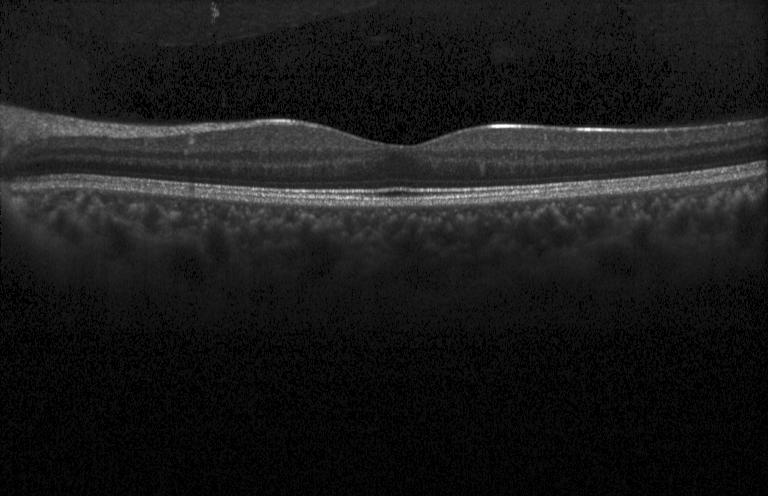 Optical coherence tomography scan · spectral-domain optical coherence tomography · acquired on a Heidelberg Spectralis · through the macula. This B-scan demonstrates no choroidal neovascularization, diabetic macular edema, or drusen.